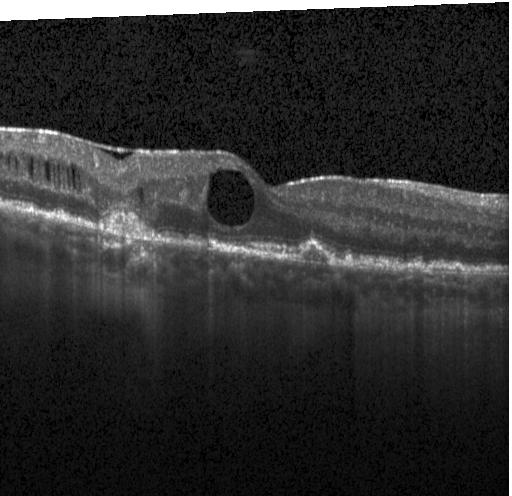
Retinal OCT cross-section — The scan shows a choroidal neovascular membrane.